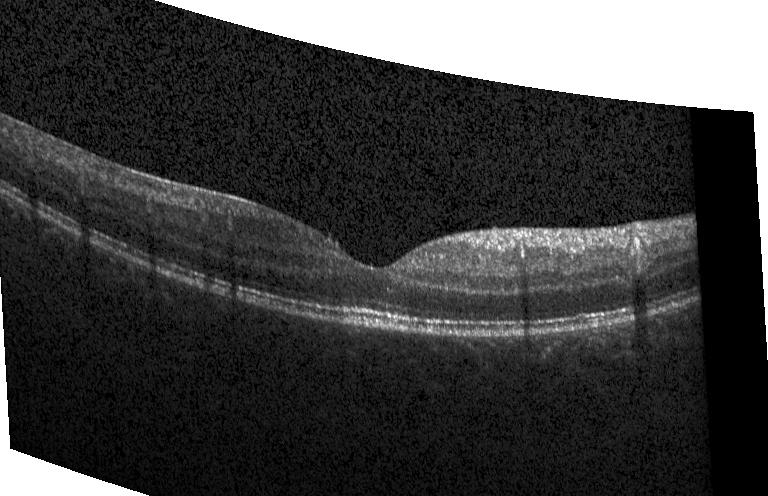
Macular OCT: no choroidal neovascularization, no diabetic macular edema, and no drusen.